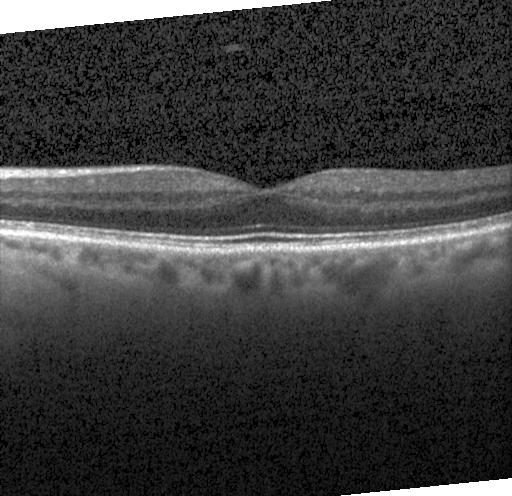
Dx: no choroidal neovascularization, diabetic macular edema, or drusen.